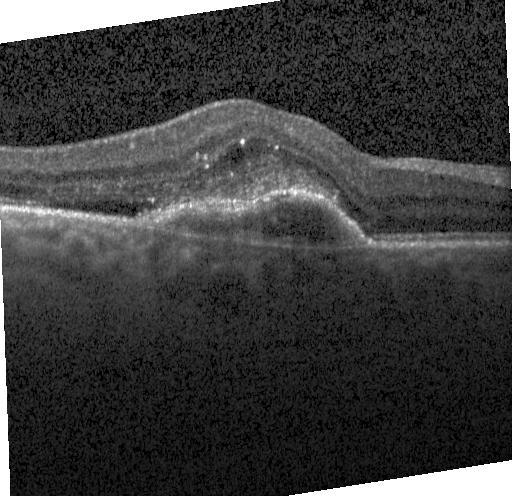 OCT B-scan
Diagnosis: choroidal neovascularization (CNV).